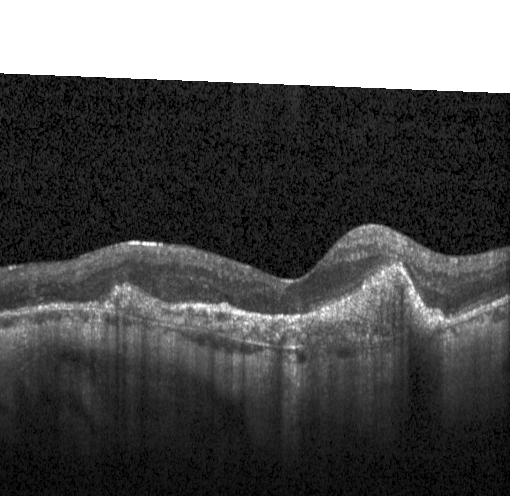
Impression: a choroidal neovascular membrane.